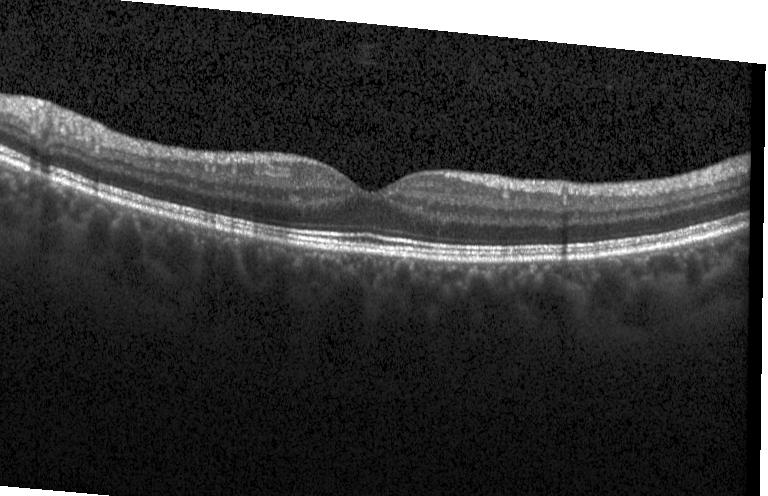 Heidelberg Spectralis · horizontal scan through the fovea · SD-OCT · optical coherence tomography B-scan. Macular OCT: no choroidal neovascularization, no diabetic macular edema, and no drusen.